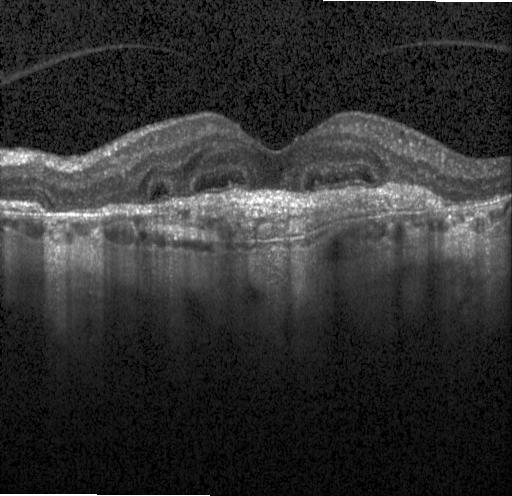
Retinal OCT B-scan; centered on the fovea; Heidelberg Spectralis. CNV.